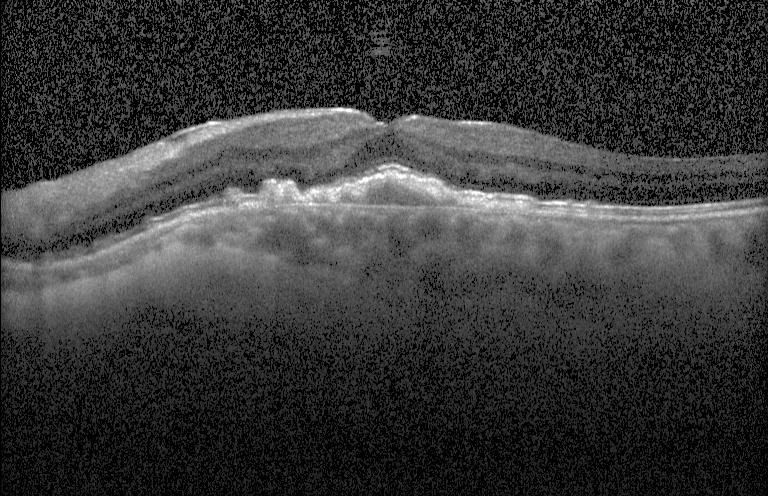
Dx: CNV.